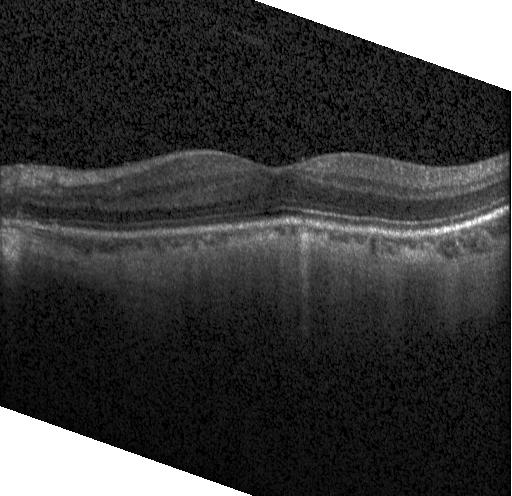

Heidelberg Spectralis OCT system. OCT line scan. Spectral-domain optical coherence tomography. Macular scan. No CNV, no DME, and no drusen.